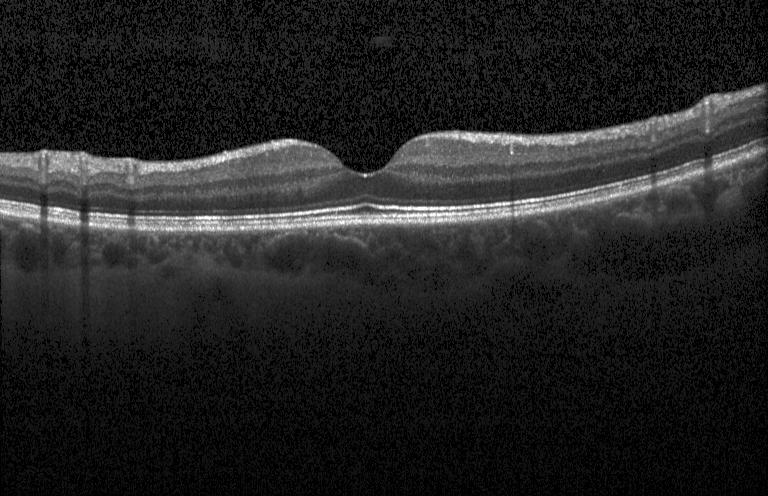

Impression: neither CNV, DME, nor drusen.